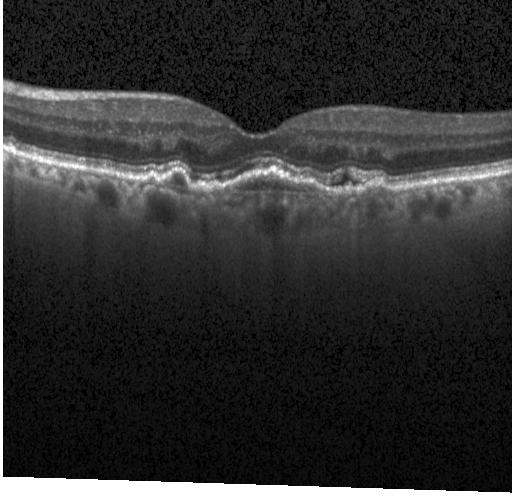

Retinal OCT cross-section · Heidelberg Spectralis · through the macula
This B-scan demonstrates choroidal neovascularization.